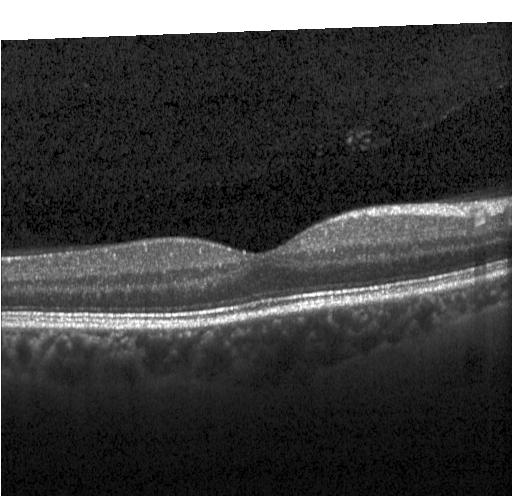 OCT line scan.
Assessment: no choroidal neovascularization, no diabetic macular edema, and no drusen.